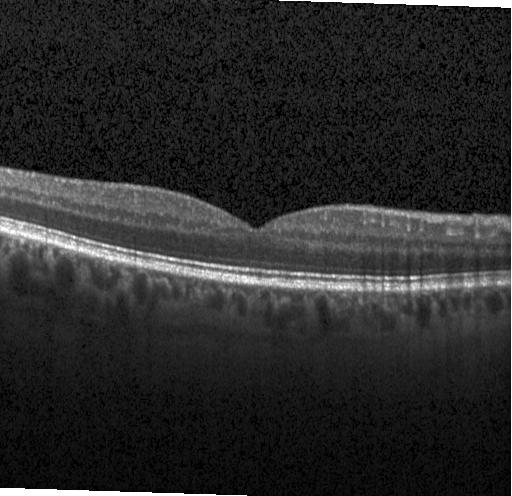
OCT line scan · Heidelberg Spectralis — Diagnosis: neither choroidal neovascularization, diabetic macular edema, nor drusen.